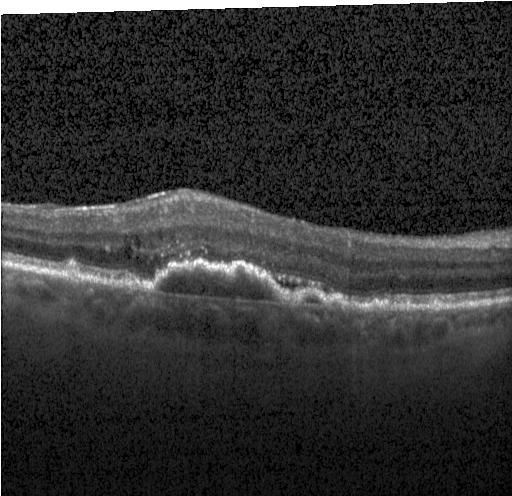
Optical coherence tomography scan; horizontal scan through the fovea; instrument: Heidelberg Spectralis.
Finding: a choroidal neovascular membrane.